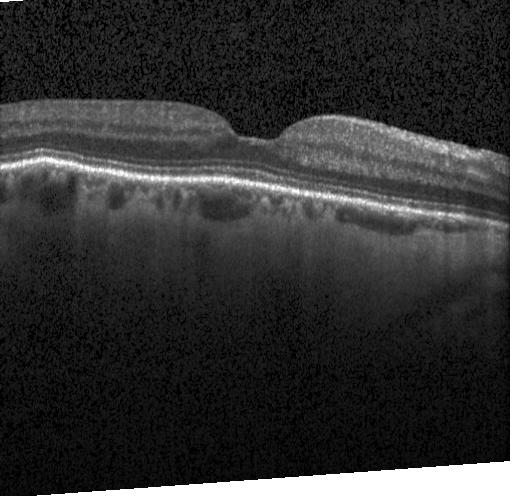 Finding: no evidence of choroidal neovascularization, diabetic macular edema, or drusen.